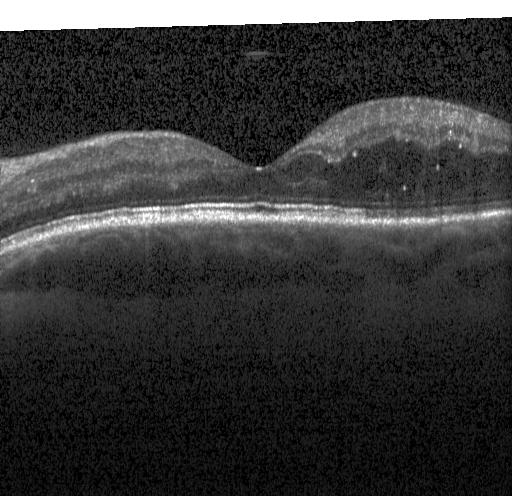 Instrument: Heidelberg Spectralis · optical coherence tomography scan · macular scan · spectral-domain optical coherence tomography. Diabetic macular edema.